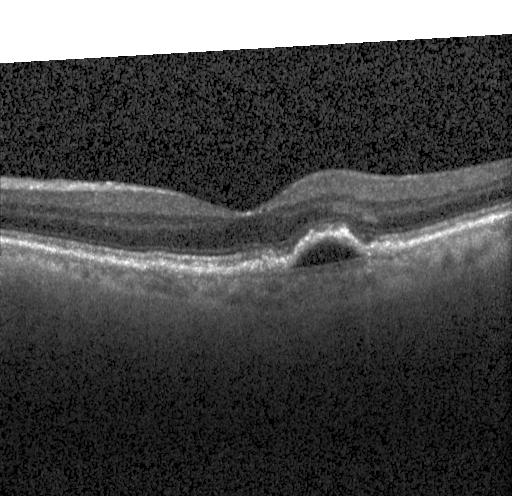 Diagnosis: a choroidal neovascular membrane.